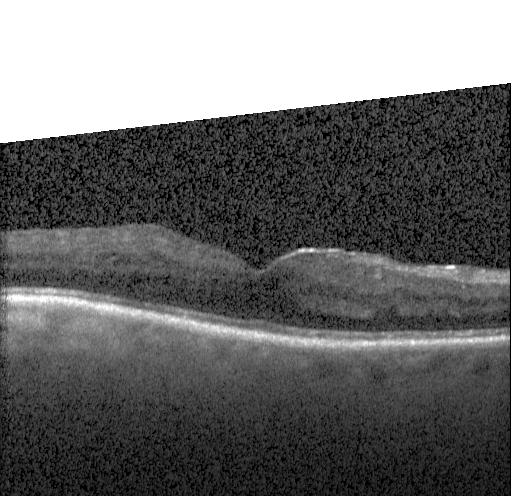 OCT finding: no evidence of choroidal neovascularization, diabetic macular edema, or drusen.